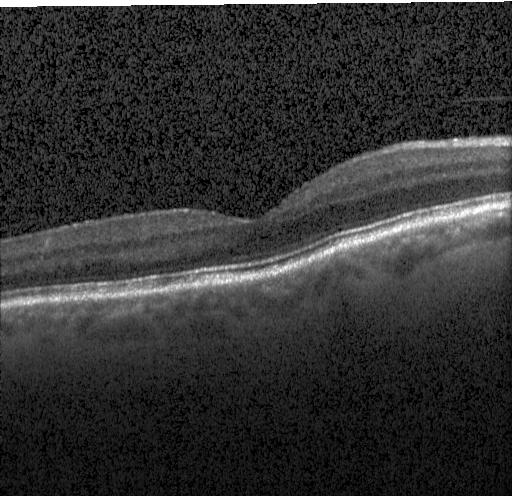

Impression: no evidence of choroidal neovascularization, diabetic macular edema, or drusen.